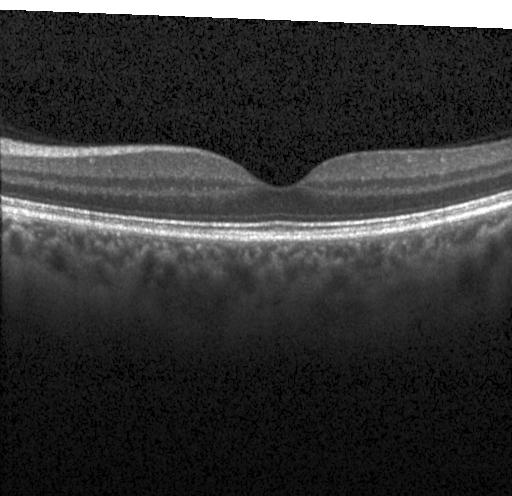 Finding: no choroidal neovascularization, no diabetic macular edema, and no drusen.